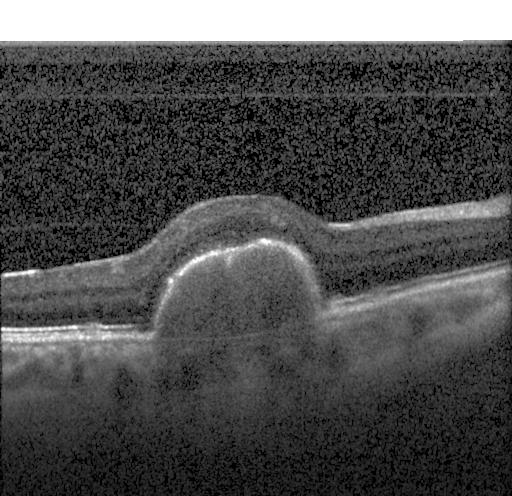 Acquired on a Heidelberg Spectralis. Optical coherence tomography B-scan — The scan shows CNV.